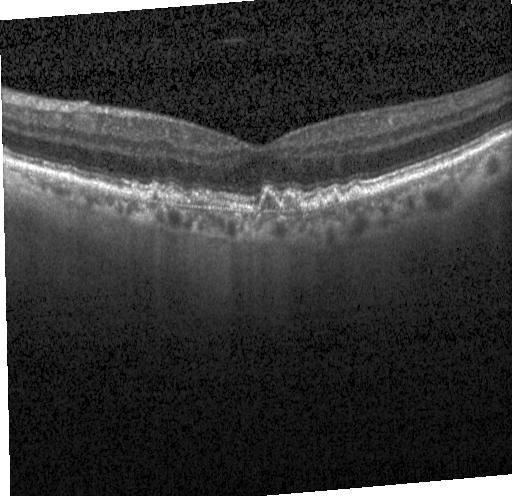
Multiple drusen.